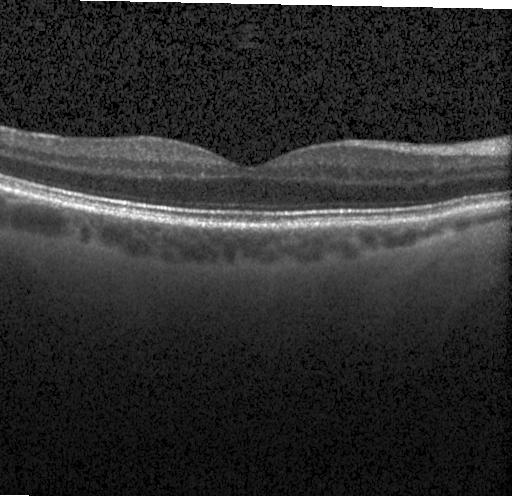
Acquired on a Heidelberg Spectralis · optical coherence tomography scan · macular scan · spectral-domain OCT.
The scan shows neither CNV, DME, nor drusen.